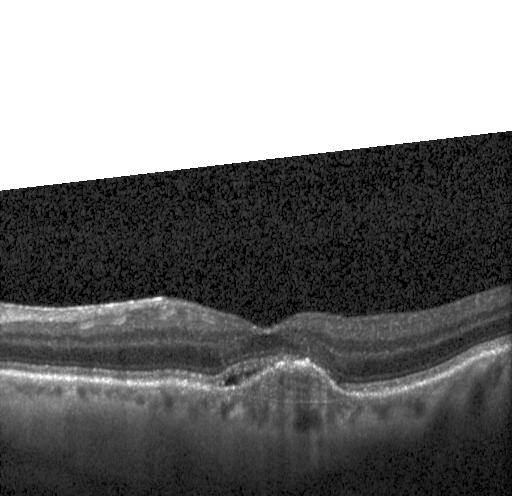

OCT B-scan showing choroidal neovascularization (CNV).